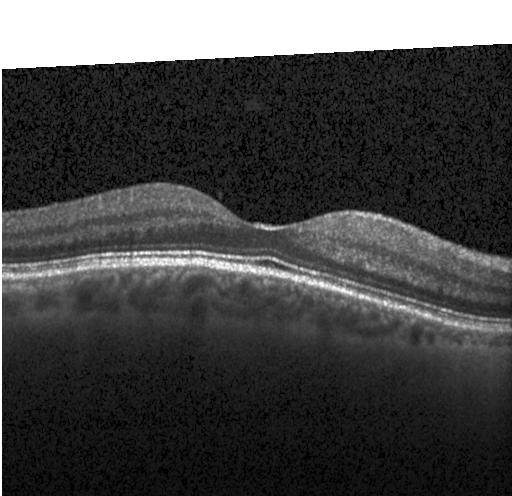
Centered on the fovea. Spectral-domain OCT. OCT line scan. Heidelberg Spectralis OCT system — The scan shows neither choroidal neovascularization, diabetic macular edema, nor drusen.